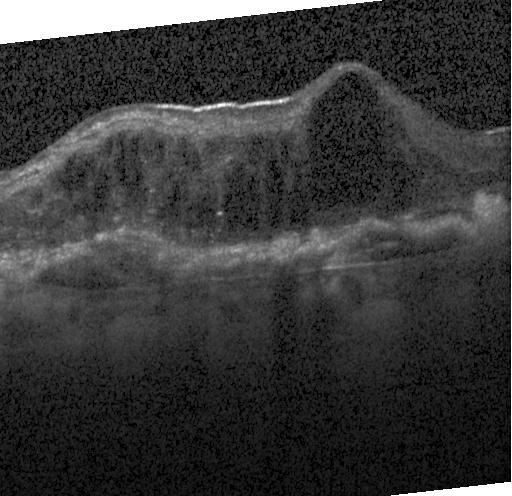 Retinal OCT cross-section · spectral-domain OCT
OCT finding: CNV.